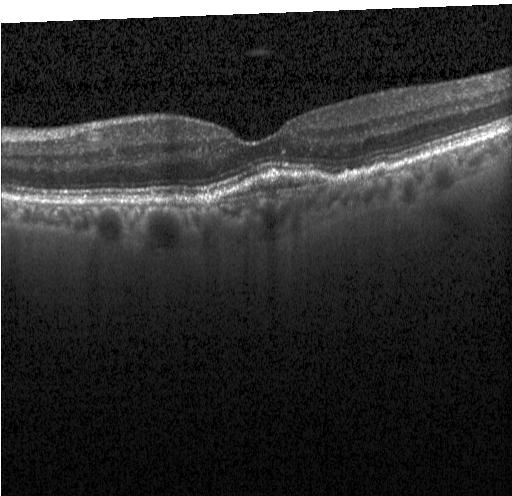 Macular OCT demonstrating choroidal neovascularization (CNV).